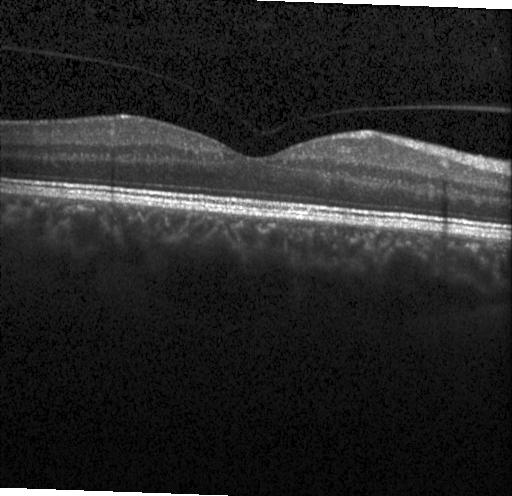

Optical coherence tomography scan.
Finding: no evidence of CNV, DME, or drusen.